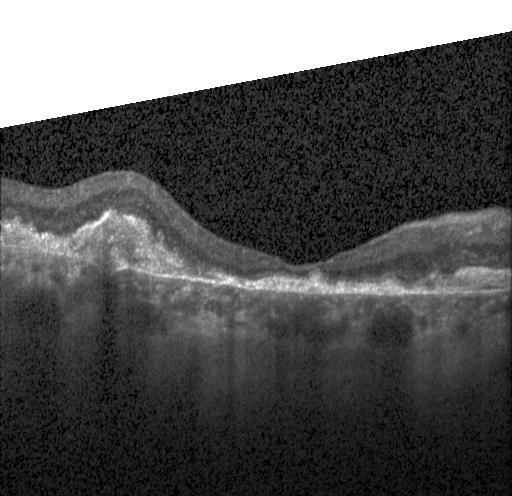
Instrument: Heidelberg Spectralis; OCT B-scan
Assessment: a choroidal neovascular membrane.